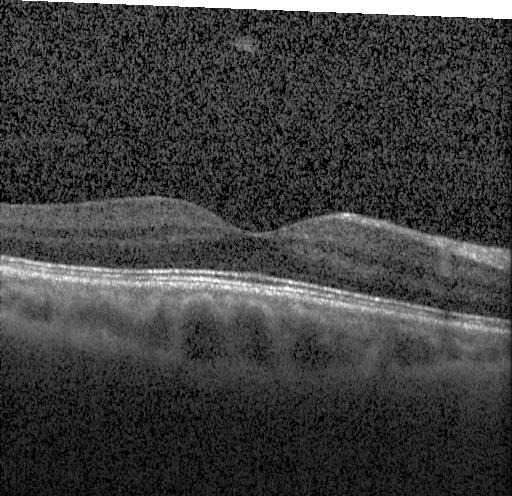
Heidelberg Spectralis · OCT line scan — Neither choroidal neovascularization, diabetic macular edema, nor drusen.